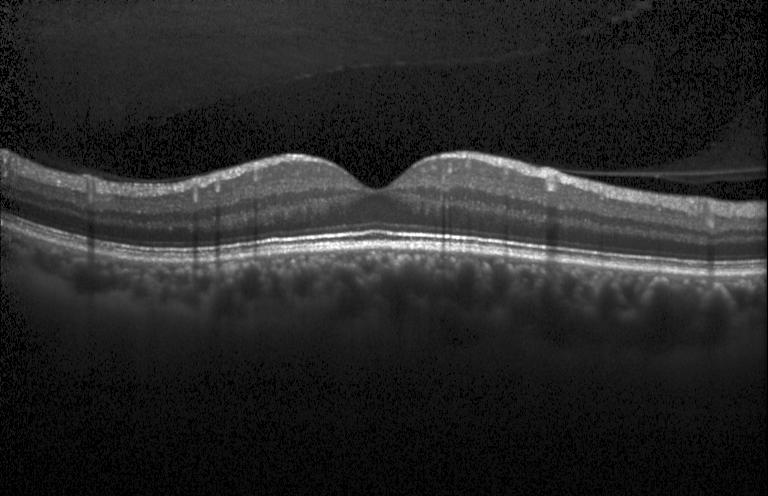
Dx: no evidence of CNV, DME, or drusen.